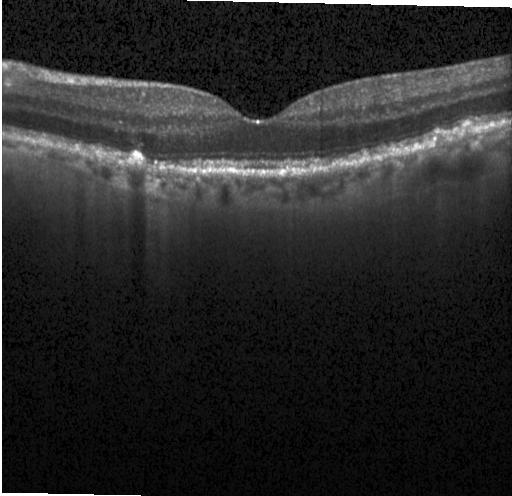
Fovea-centered, spectral-domain optical coherence tomography, retinal OCT cross-section
Sub-RPE drusenoid deposits.